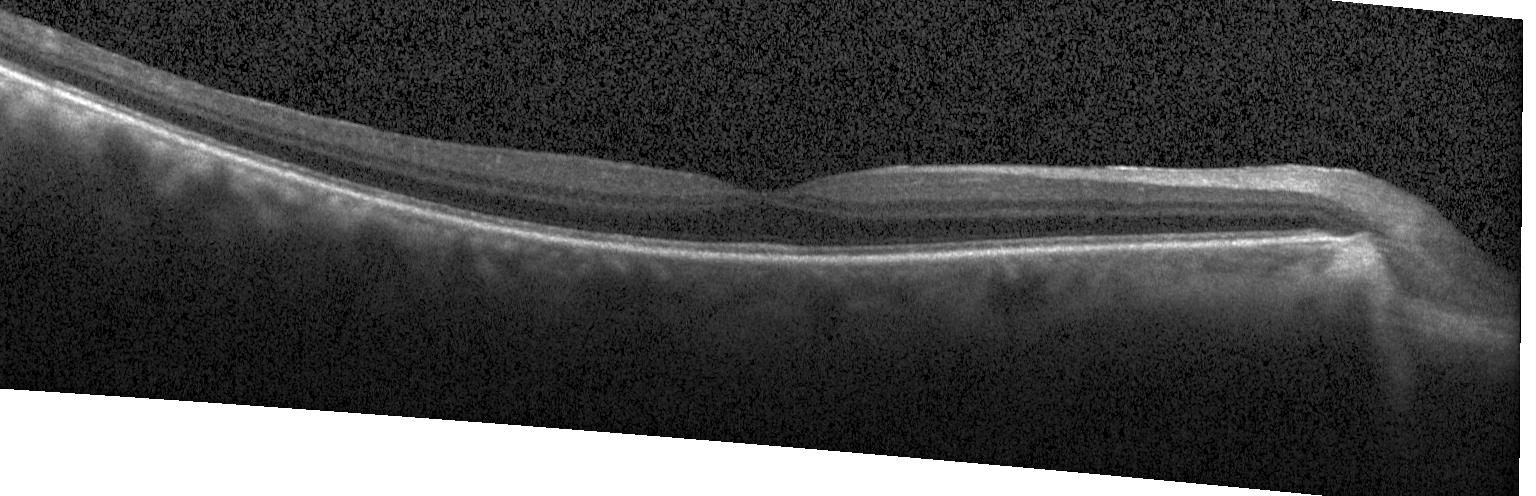
Impression: no CNV, DME, or drusen.